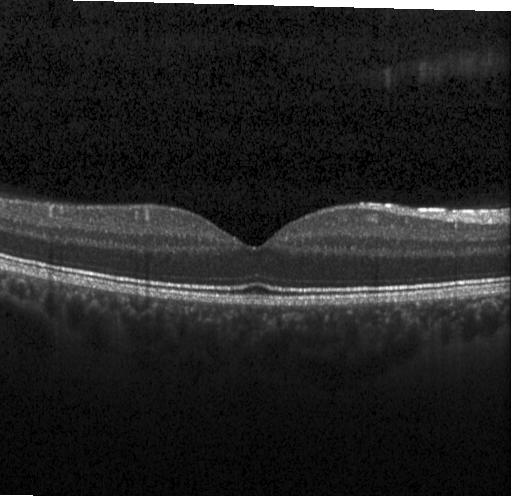
Retinal OCT B-scan. SD-OCT. Macular scan. Heidelberg Spectralis OCT system. The scan shows no choroidal neovascularization, no diabetic macular edema, and no drusen.